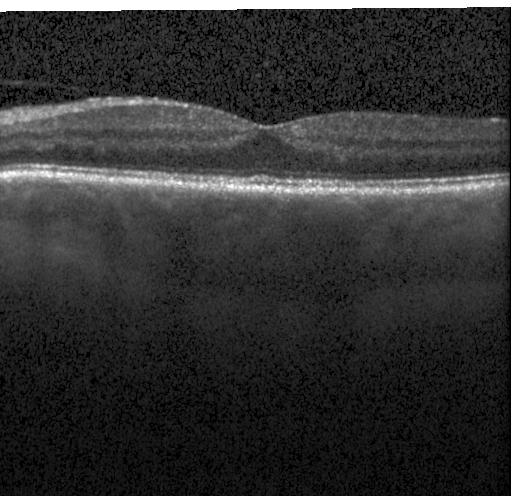

Optical coherence tomography scan. OCT finding: no CNV, DME, or drusen.